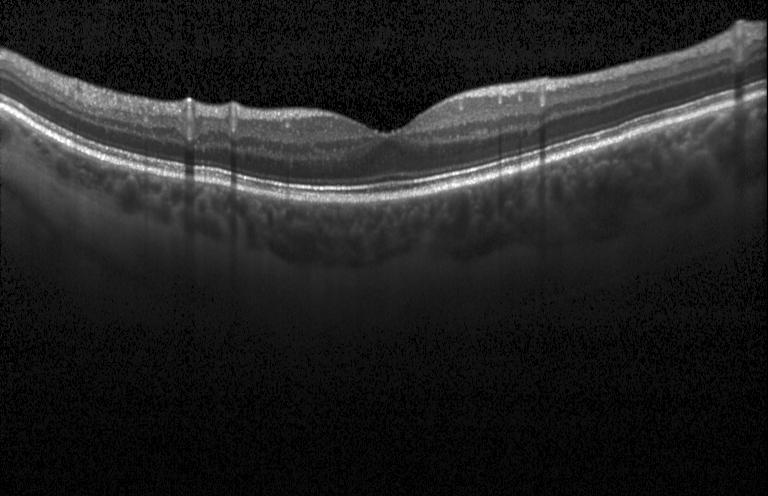
Dx: no CNV, no DME, and no drusen.